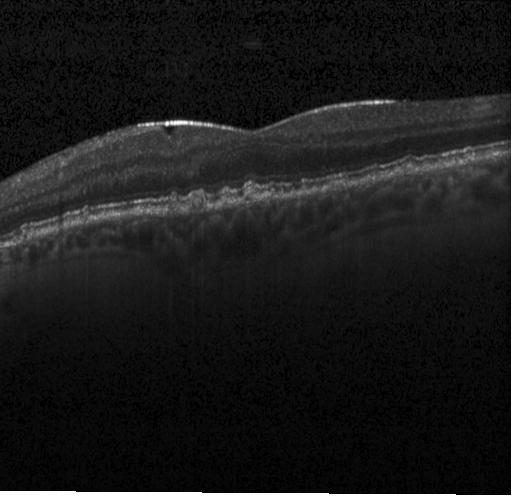 OCT scan showing drusen.